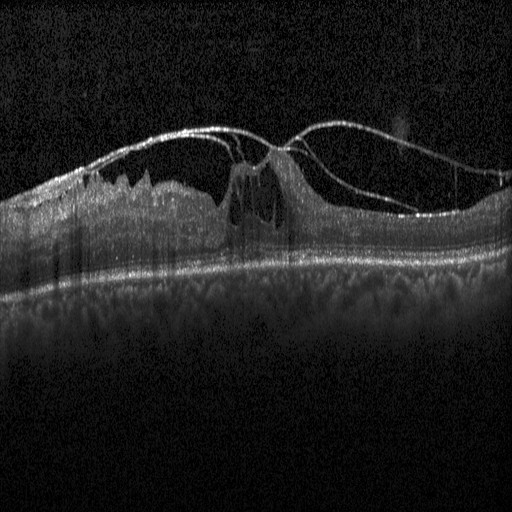

Spectral-domain optical coherence tomography, retinal OCT B-scan
OCT finding: diabetic macular edema.